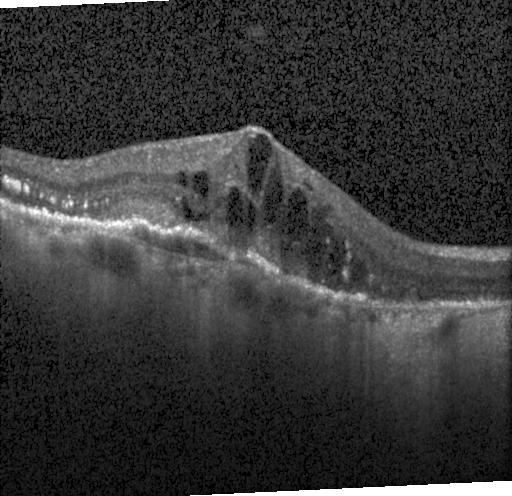

Spectral-domain optical coherence tomography · OCT line scan
Finding: a choroidal neovascular membrane.